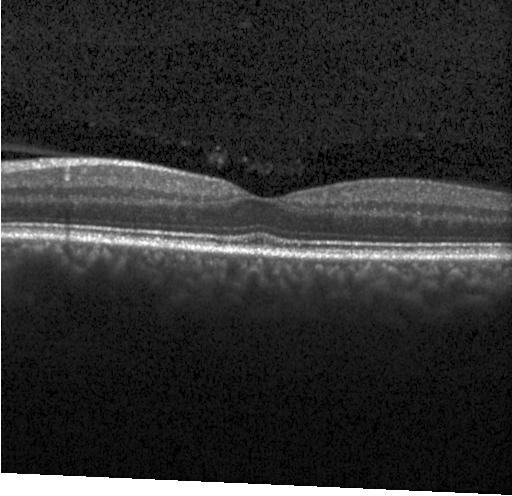
Impression: no choroidal neovascularization, diabetic macular edema, or drusen.